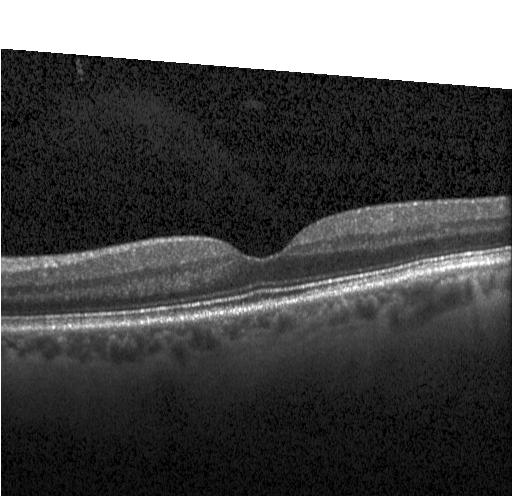

OCT line scan
Impression: neither choroidal neovascularization, diabetic macular edema, nor drusen.